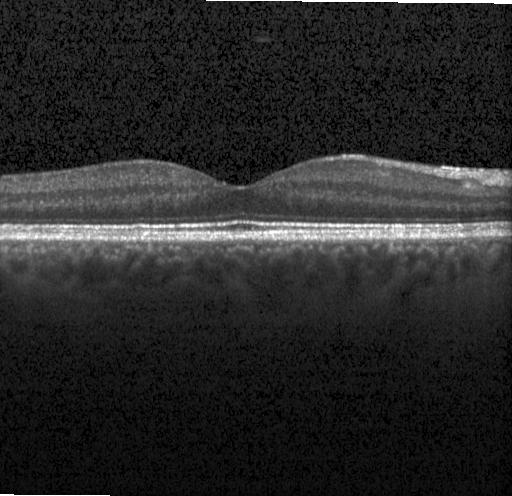
OCT B-scan; SD-OCT. Impression: no choroidal neovascularization, diabetic macular edema, or drusen.